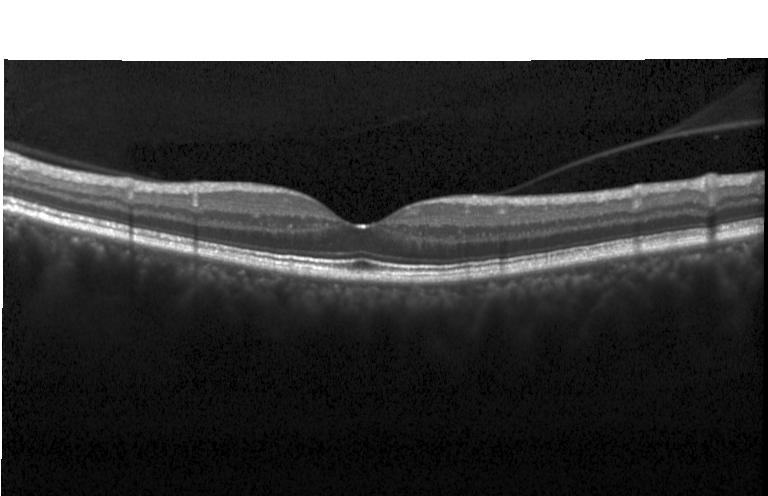
Macular OCT: neither choroidal neovascularization, diabetic macular edema, nor drusen.